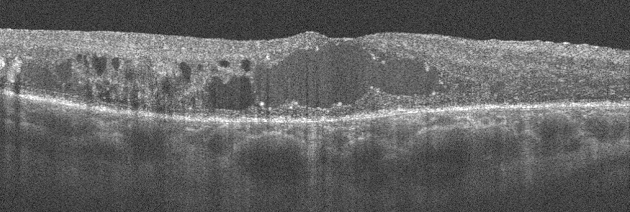

OCT scan showing DME.